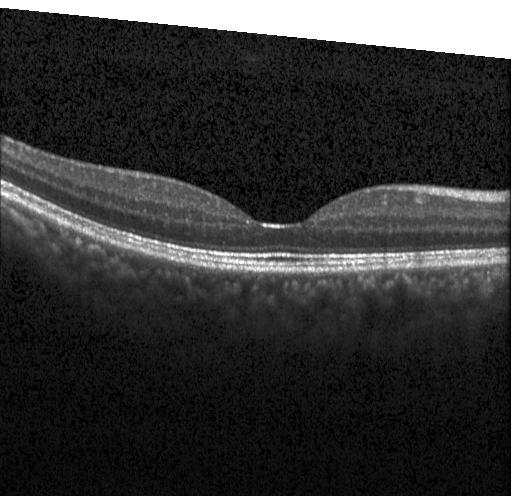
Fovea-centered; optical coherence tomography B-scan
Neither choroidal neovascularization, diabetic macular edema, nor drusen.